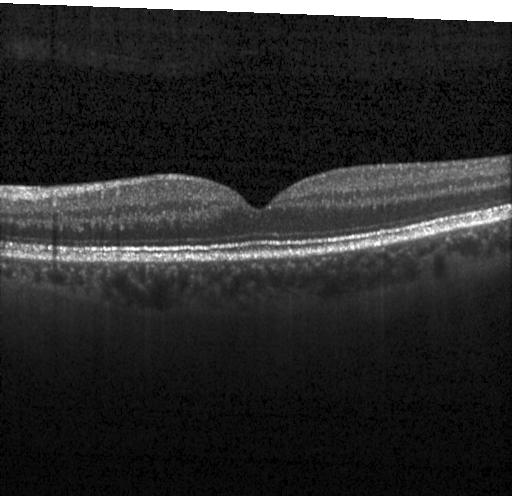

Optical coherence tomography B-scan, macular scan — OCT finding: no choroidal neovascularization, diabetic macular edema, or drusen.